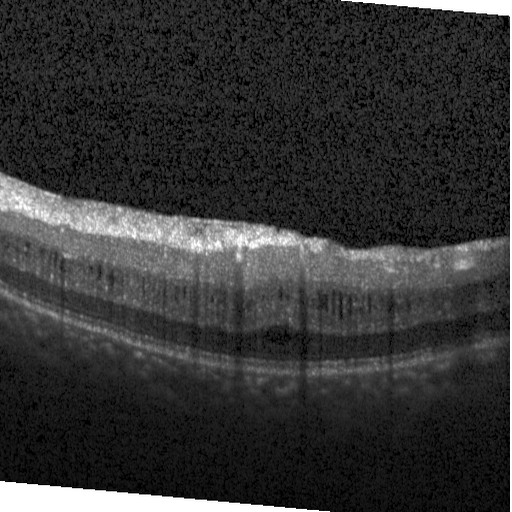

Diagnosis: diabetic macular edema.